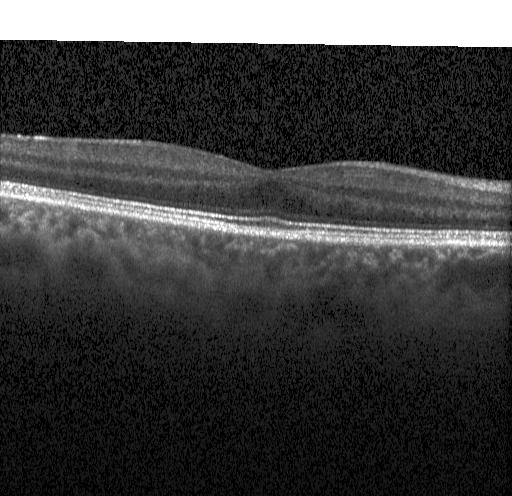
Retinal OCT cross-section · spectral-domain OCT
Impression: no evidence of CNV, DME, or drusen.